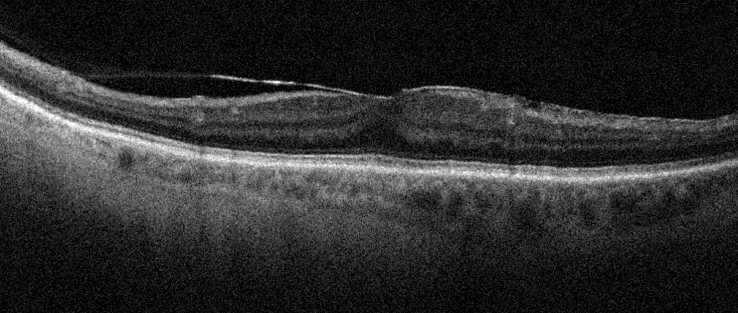 Retinal OCT B-scan. Macular scan. Acquired on an Optovue Avanti RTVue XR.
OCT finding: ERM.